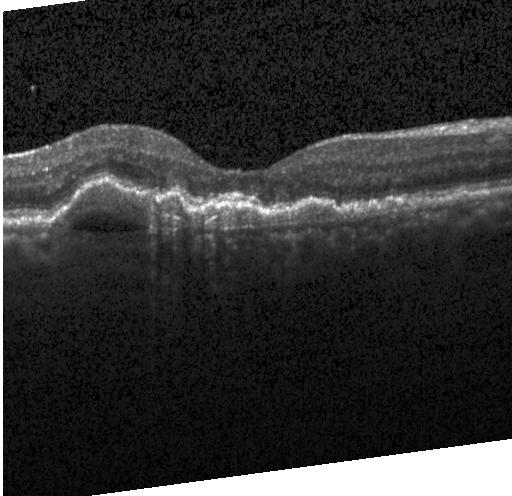

Instrument: Heidelberg Spectralis. Retinal OCT B-scan — OCT finding: a choroidal neovascular membrane.